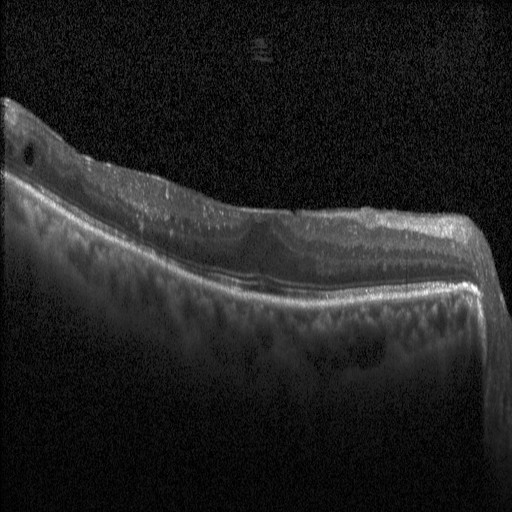 OCT B-scan — Diagnosis: diabetic macular edema (DME).